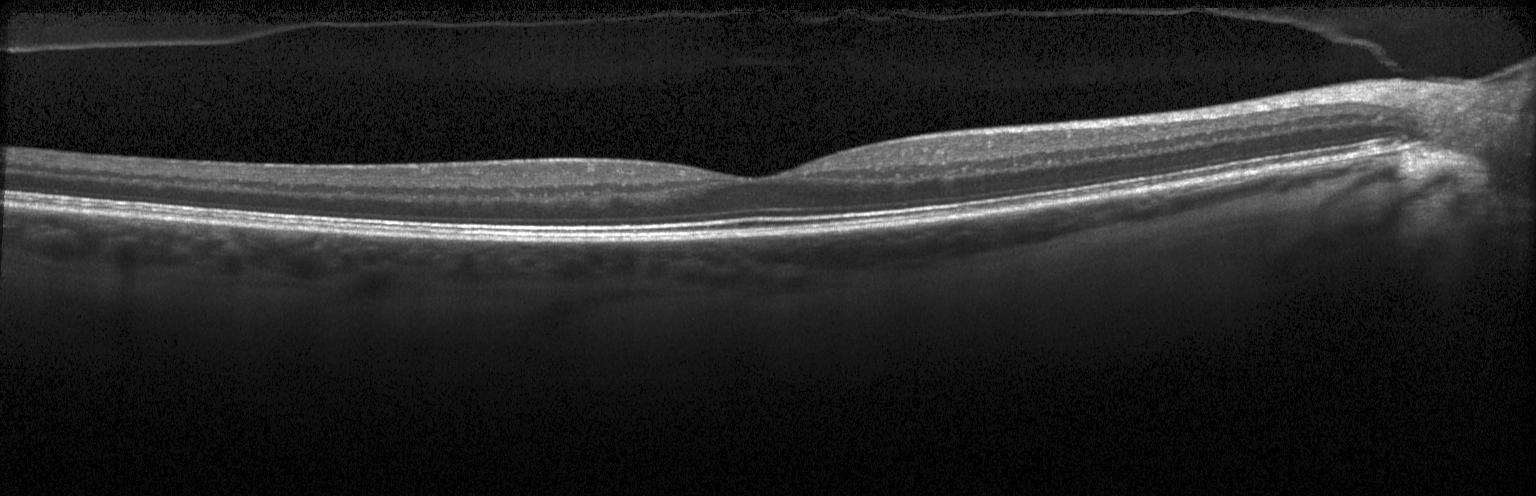

This B-scan demonstrates no choroidal neovascularization, diabetic macular edema, or drusen.